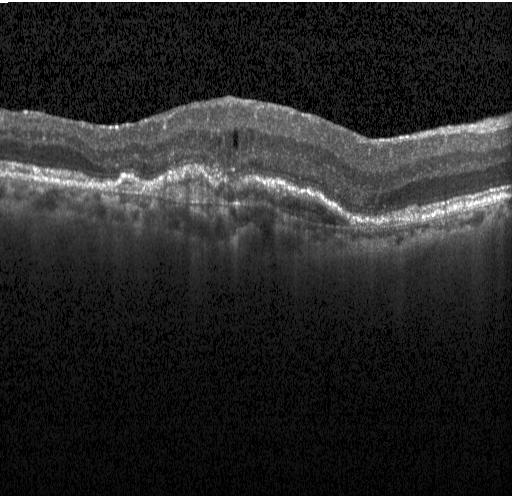
Heidelberg Spectralis OCT system. Retinal OCT cross-section — Finding: CNV.